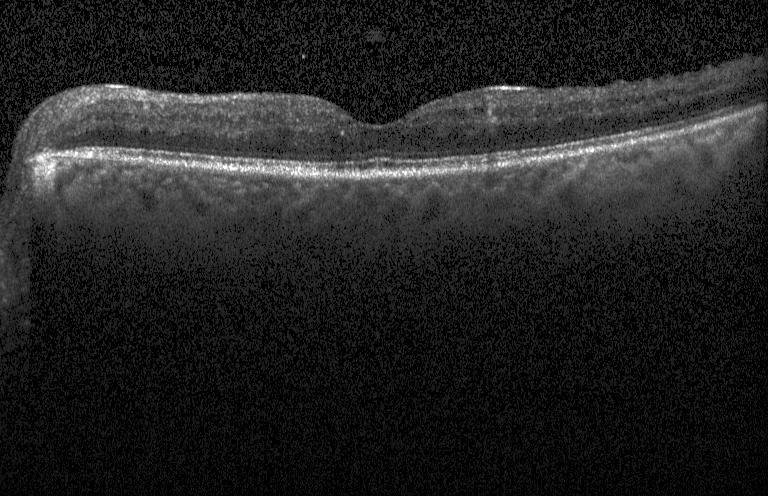
Spectral-domain OCT B-scan: no CNV, no DME, and no drusen.